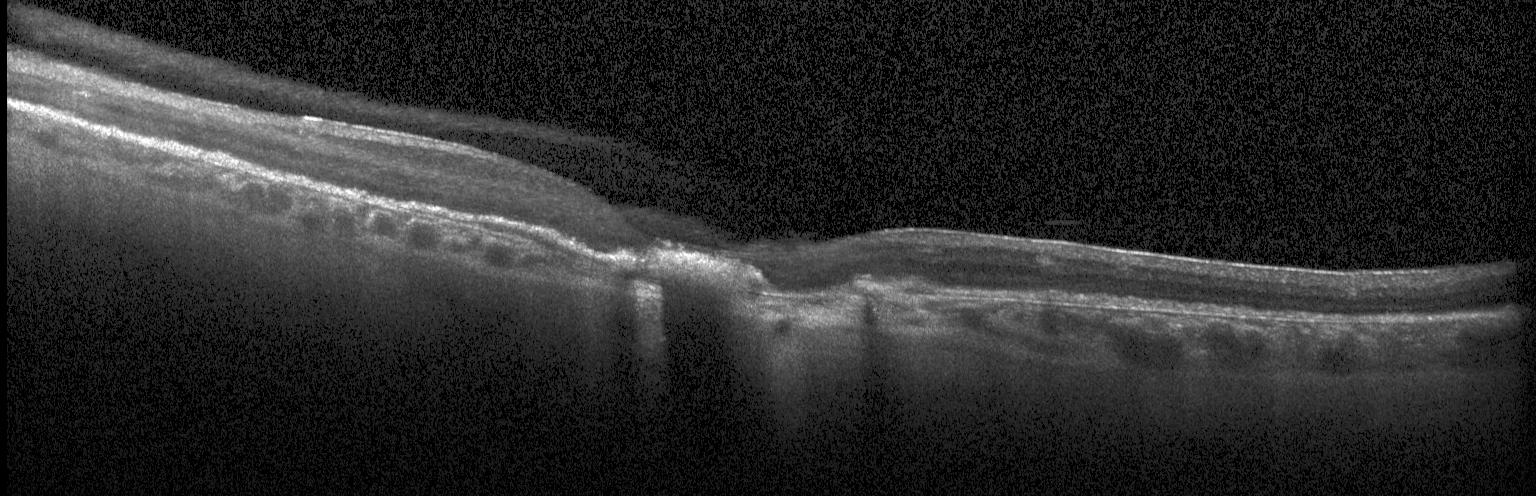
Diagnosis: a choroidal neovascular membrane.